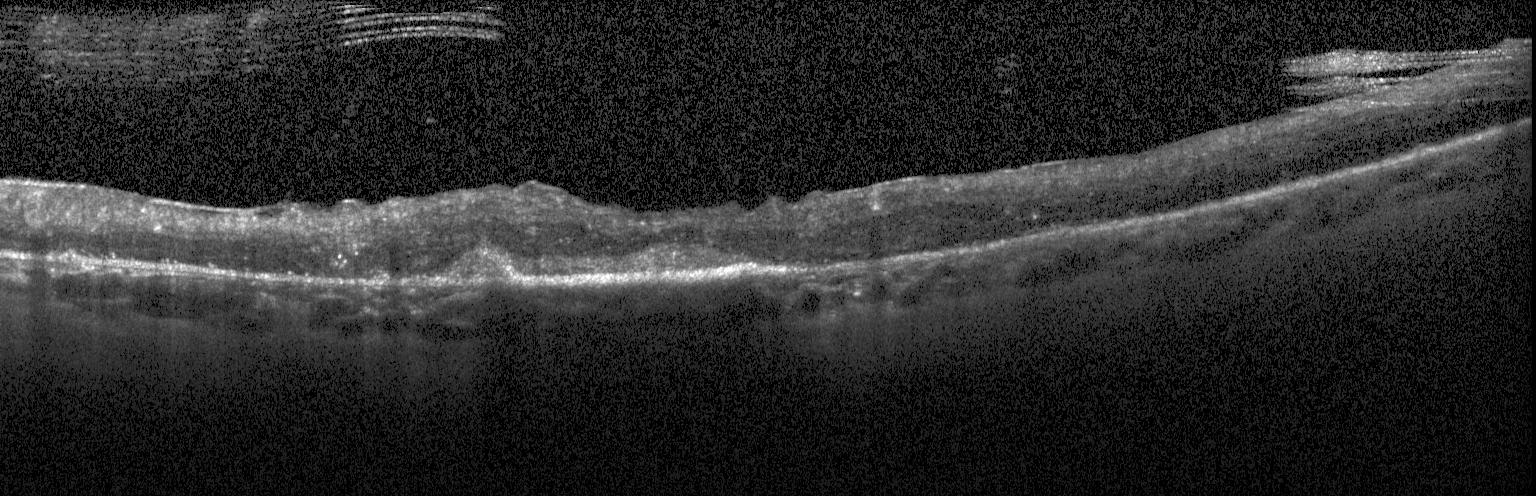
Macular scan; optical coherence tomography B-scan; spectral-domain OCT; instrument: Heidelberg Spectralis. Assessment: a choroidal neovascular membrane.